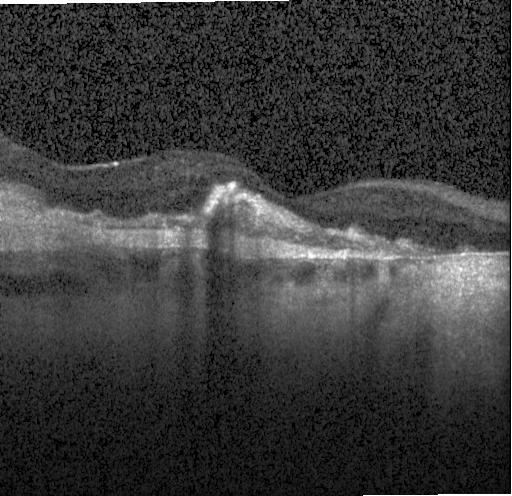

Macular scan. Instrument: Heidelberg Spectralis. Retinal OCT B-scan.
Diagnosis: choroidal neovascularization (CNV).